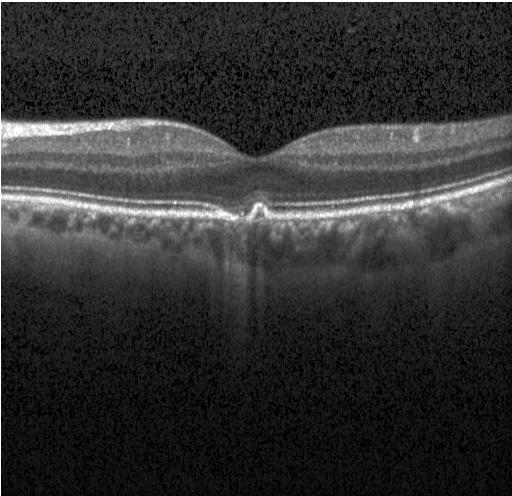
Heidelberg Spectralis OCT system · retinal OCT B-scan.
Impression: drusen.